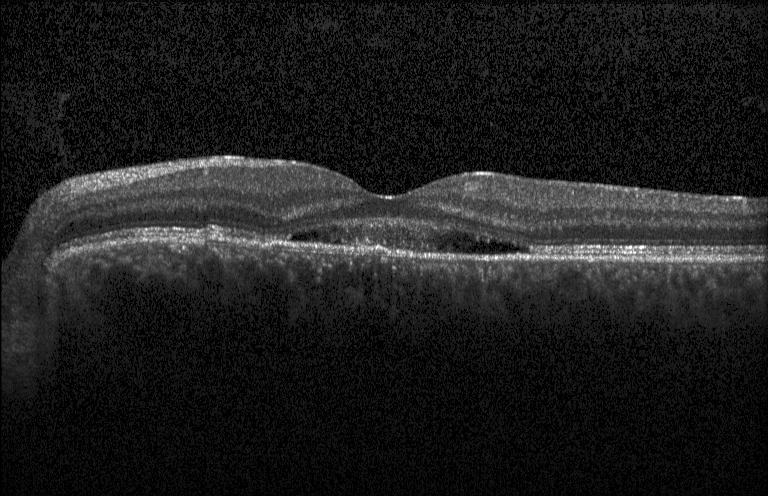 Optical coherence tomography B-scan — This B-scan demonstrates a choroidal neovascular membrane.